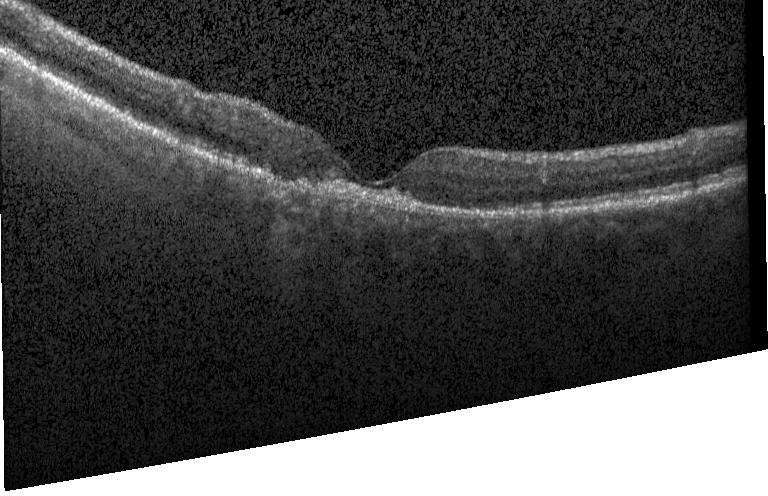 This B-scan demonstrates a choroidal neovascular membrane.